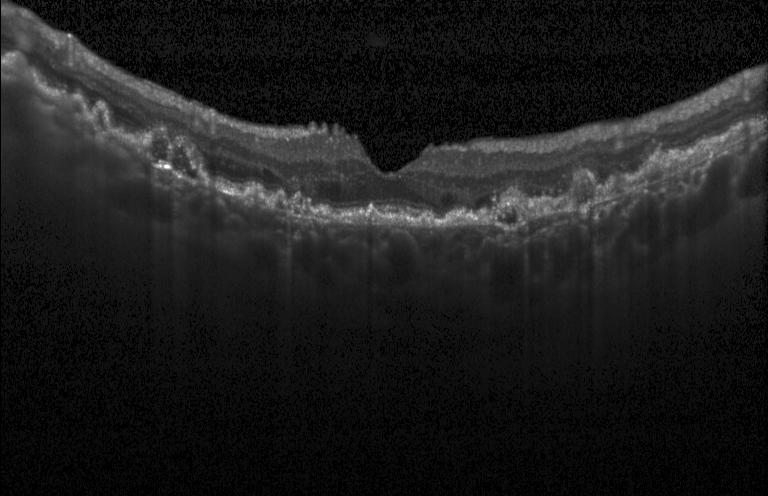 Impression: a choroidal neovascular membrane.